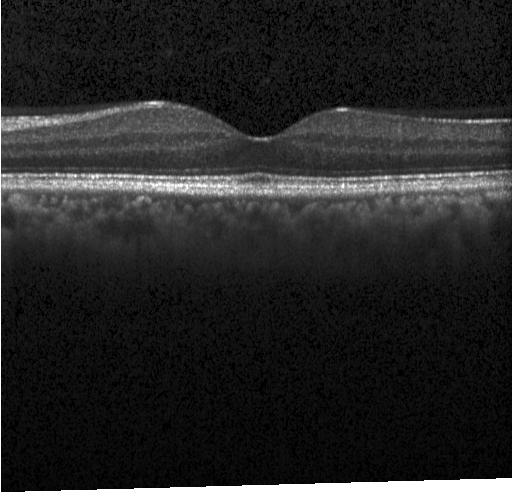

This B-scan demonstrates no choroidal neovascularization, no diabetic macular edema, and no drusen.